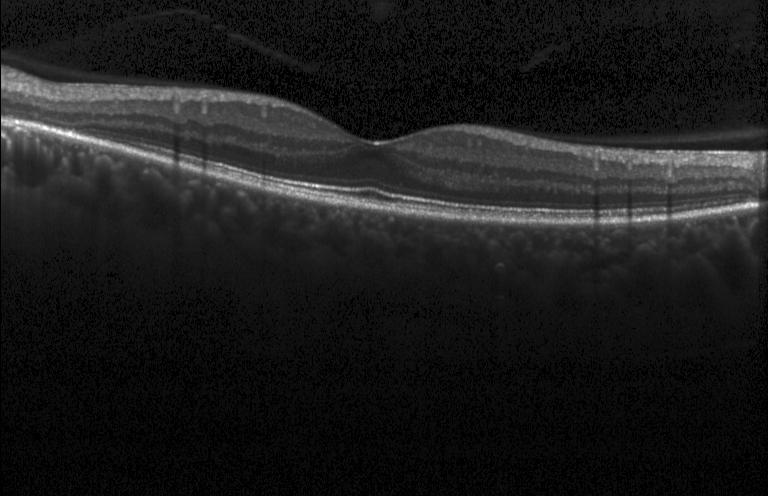
Dx: no evidence of choroidal neovascularization, diabetic macular edema, or drusen.